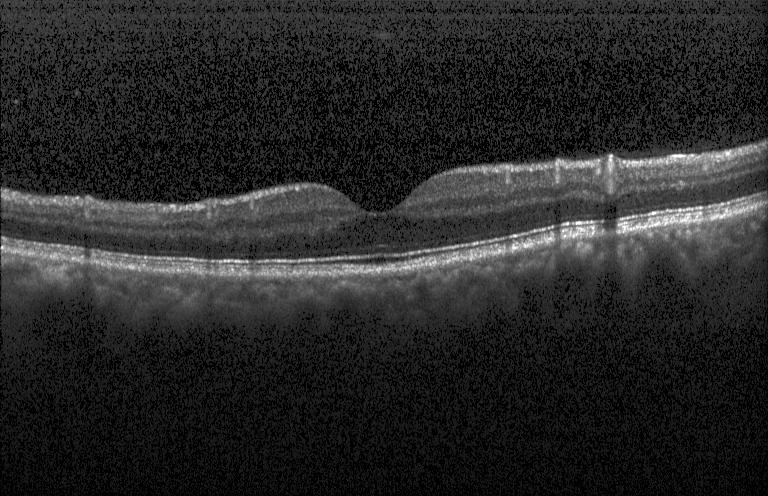 Optical coherence tomography B-scan; through the macula; spectral-domain optical coherence tomography; instrument: Heidelberg Spectralis — Diagnosis: no choroidal neovascularization, diabetic macular edema, or drusen.